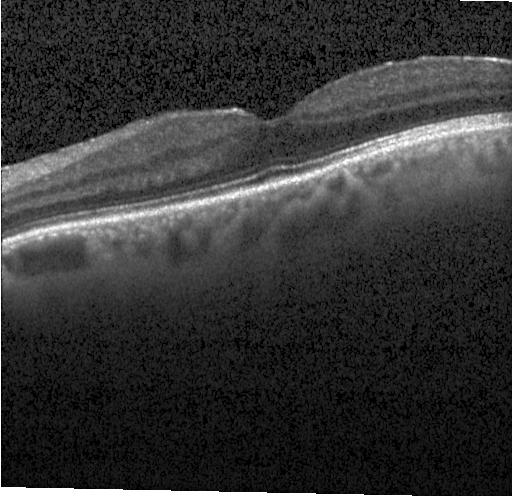 Macular OCT: no evidence of CNV, DME, or drusen.